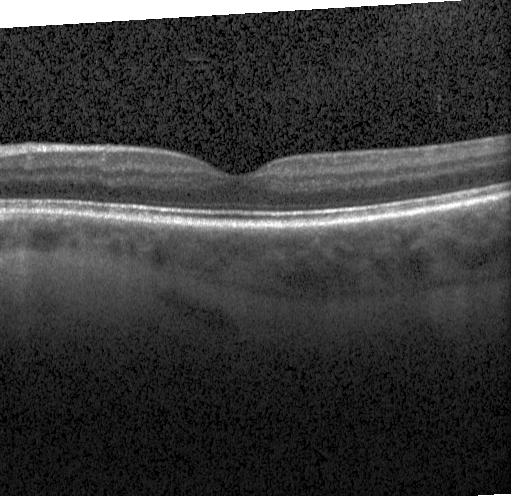 Acquired on a Heidelberg Spectralis · through the macula · optical coherence tomography B-scan — This B-scan demonstrates no choroidal neovascularization, no diabetic macular edema, and no drusen.